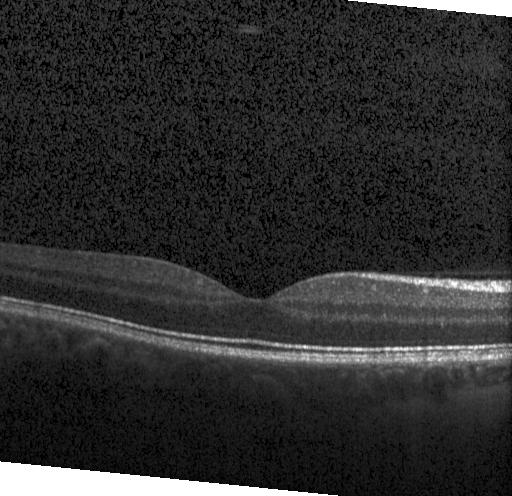
Retinal OCT B-scan
Diagnosis: no evidence of CNV, DME, or drusen.